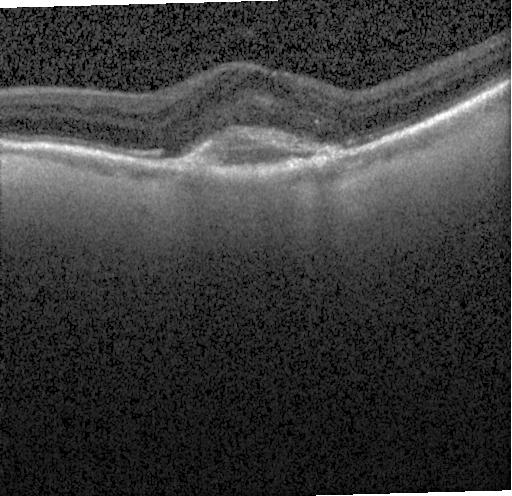

OCT B-scan showing a choroidal neovascular membrane.